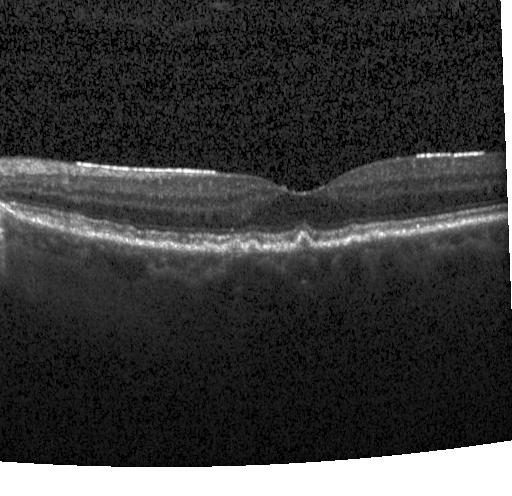
Spectral-domain OCT; retinal OCT cross-section; Heidelberg Spectralis OCT system; centered on the fovea — Assessment: multiple drusen.